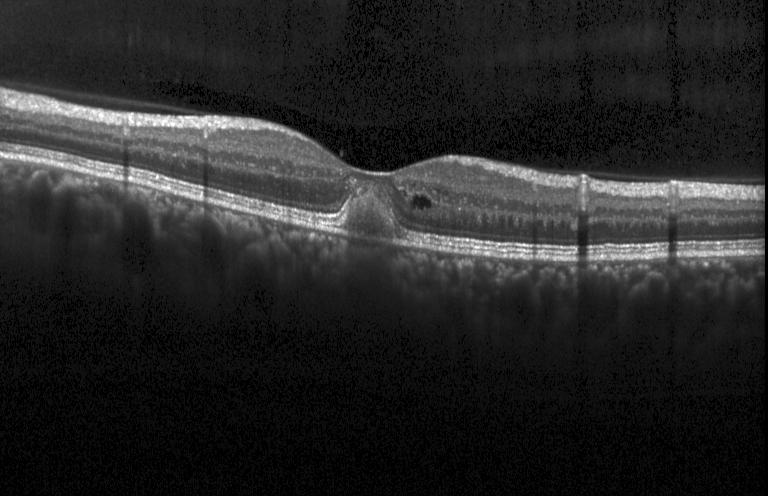 Optical coherence tomography B-scan, SD-OCT
Impression: a choroidal neovascular membrane.